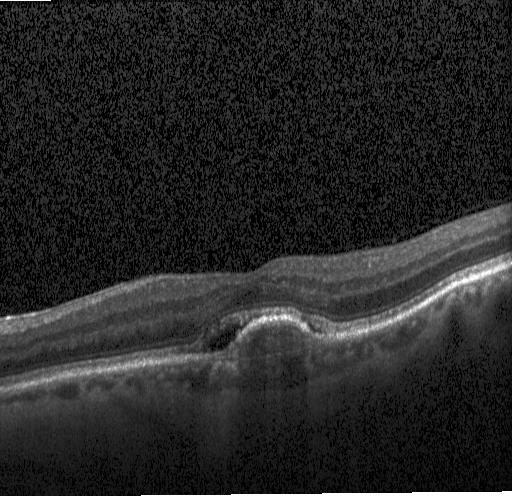

A choroidal neovascular membrane.